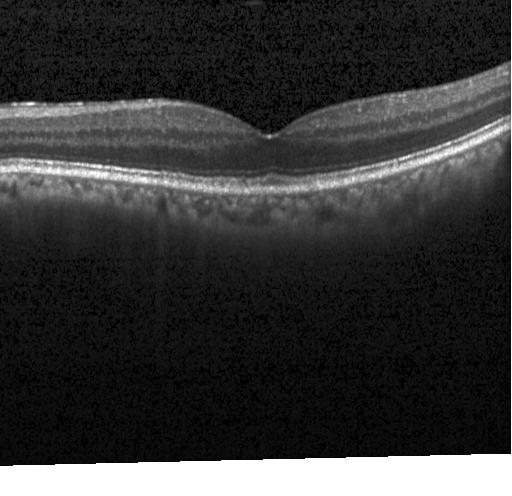

OCT scan showing neither choroidal neovascularization, diabetic macular edema, nor drusen.